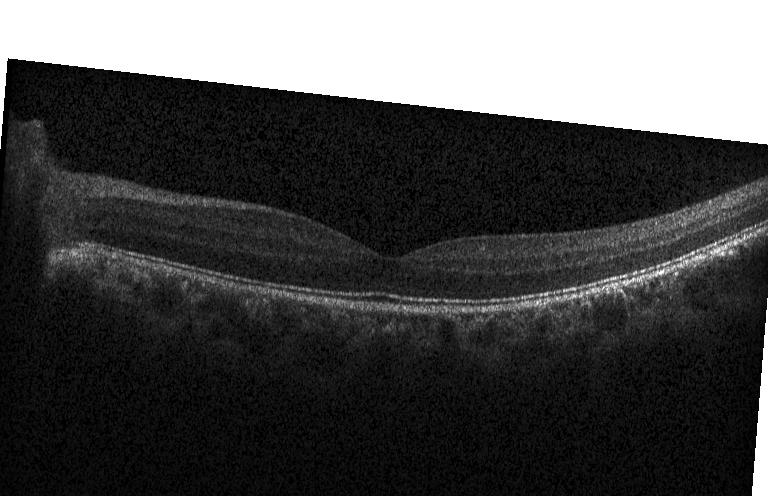

OCT line scan, SD-OCT, Heidelberg Spectralis, macular scan — The scan shows no choroidal neovascularization, no diabetic macular edema, and no drusen.